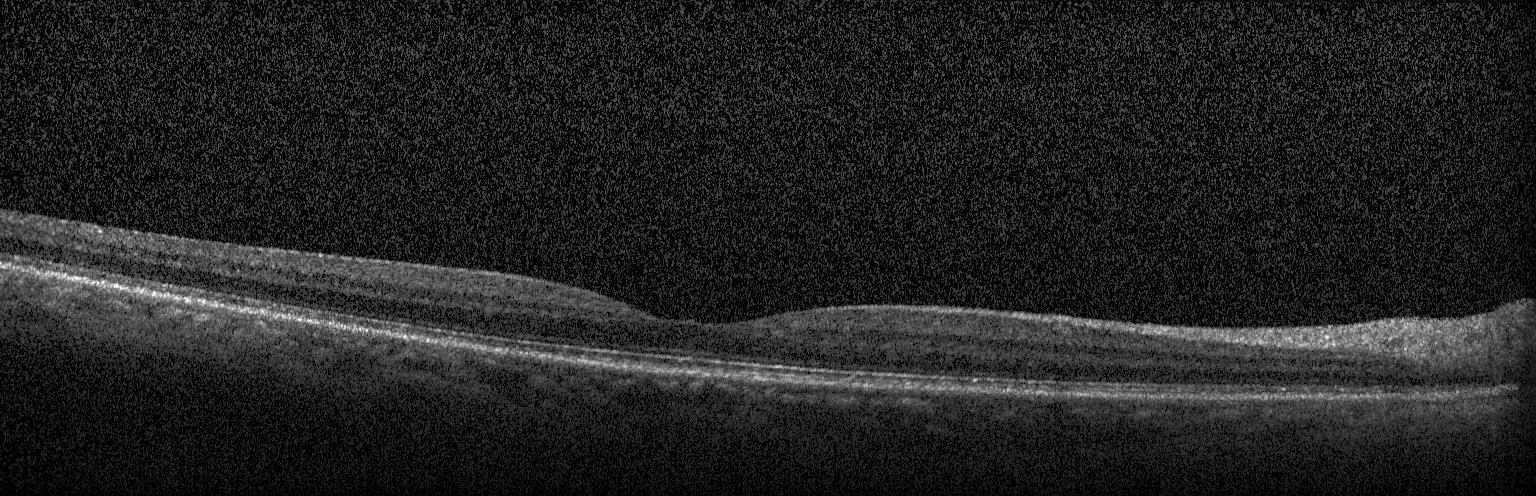

Finding: no choroidal neovascularization, diabetic macular edema, or drusen.